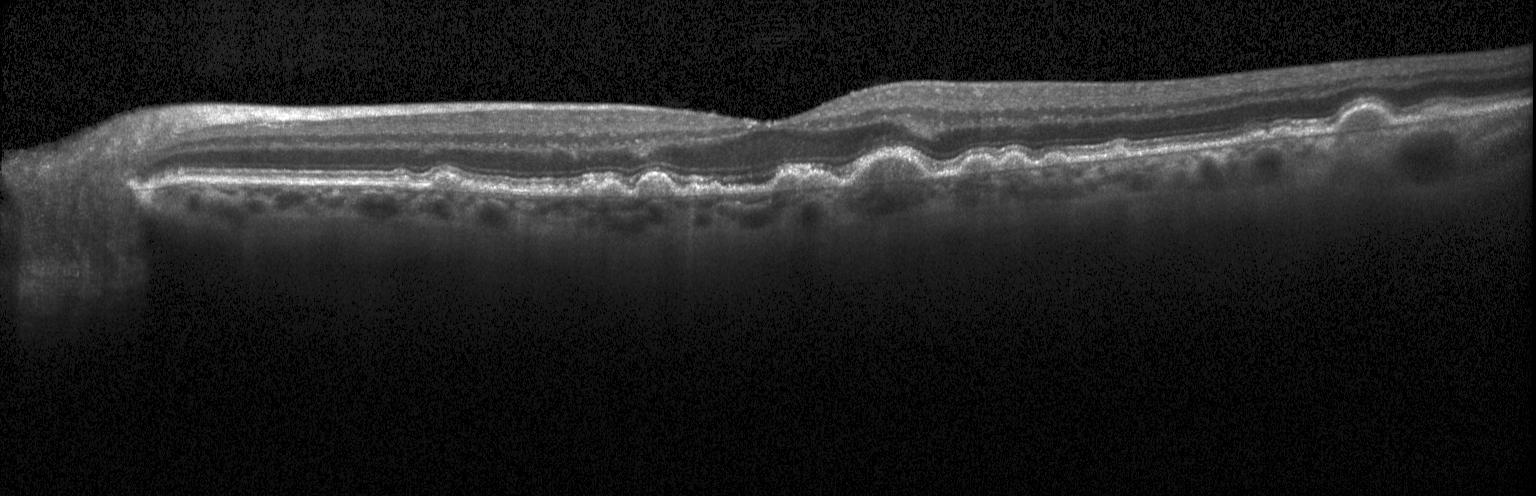

Diagnosis: sub-RPE drusenoid deposits.